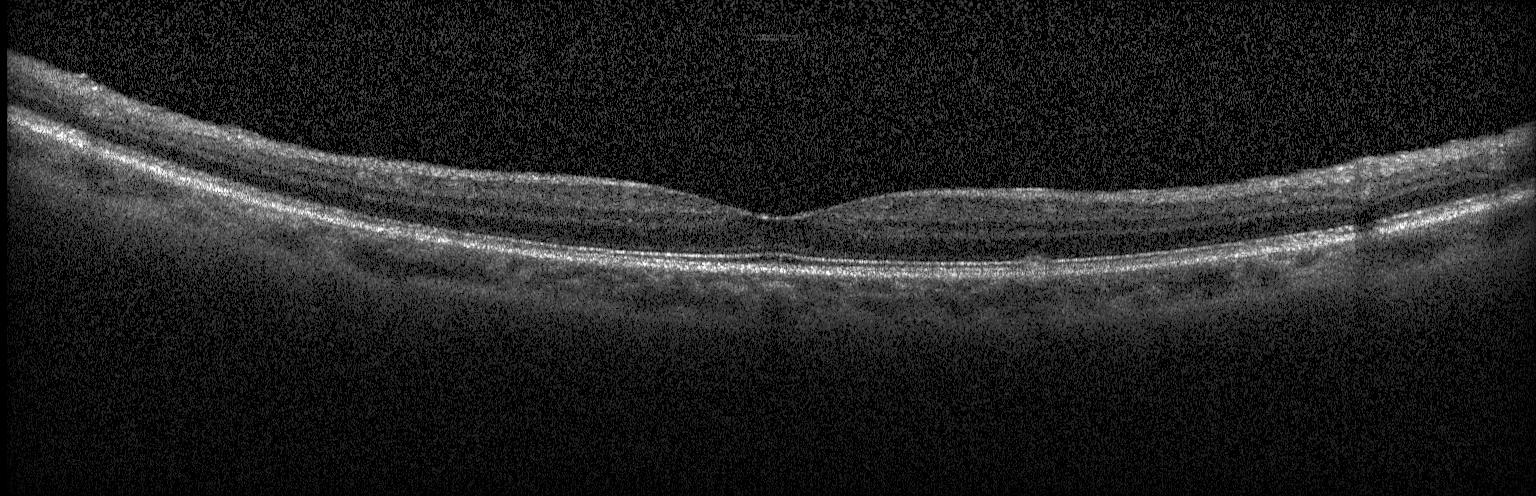

Horizontal scan through the fovea. Optical coherence tomography B-scan. Spectral-domain OCT. Instrument: Heidelberg Spectralis. Diagnosis: no choroidal neovascularization, no diabetic macular edema, and no drusen.